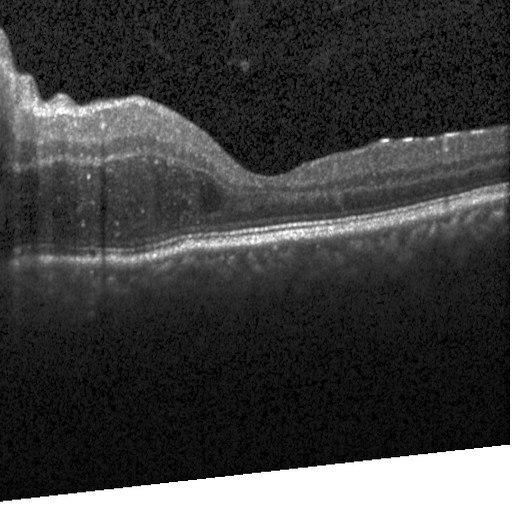 Finding: diabetic macular edema (DME).